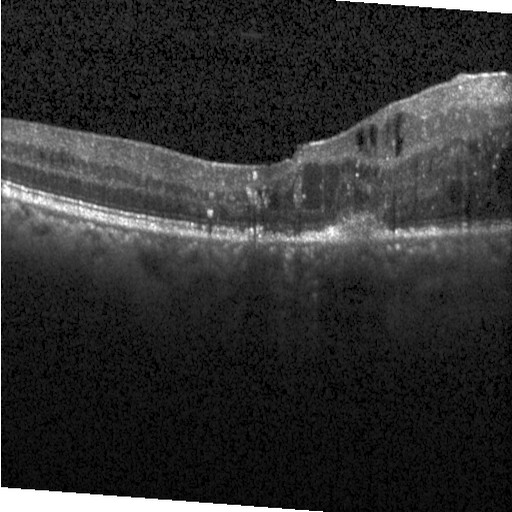
OCT finding: diabetic macular edema.